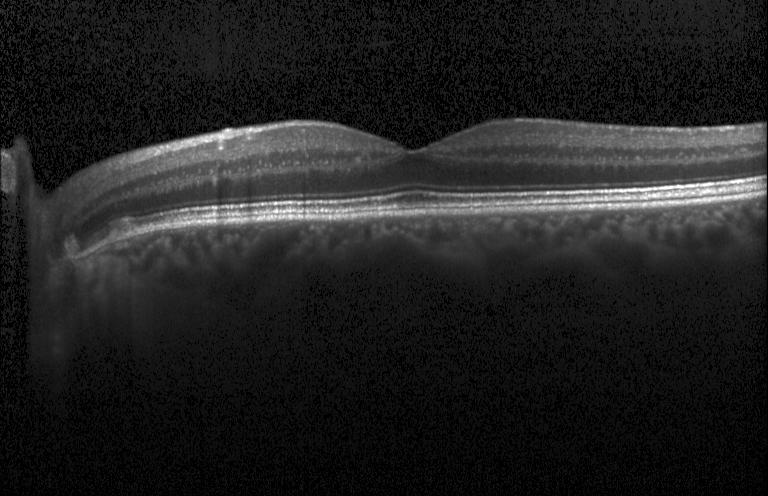 Retinal OCT cross-section · Heidelberg Spectralis — OCT finding: no choroidal neovascularization, diabetic macular edema, or drusen.